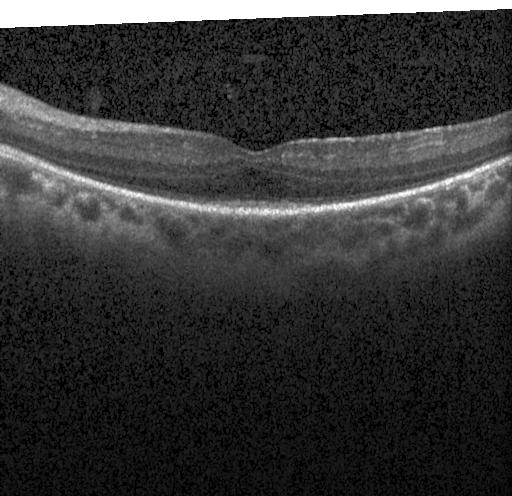
OCT finding: no evidence of choroidal neovascularization, diabetic macular edema, or drusen.